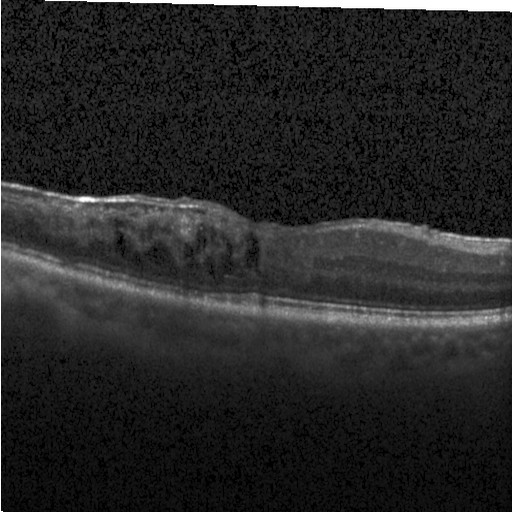 Diagnosis: diabetic macular edema (DME).